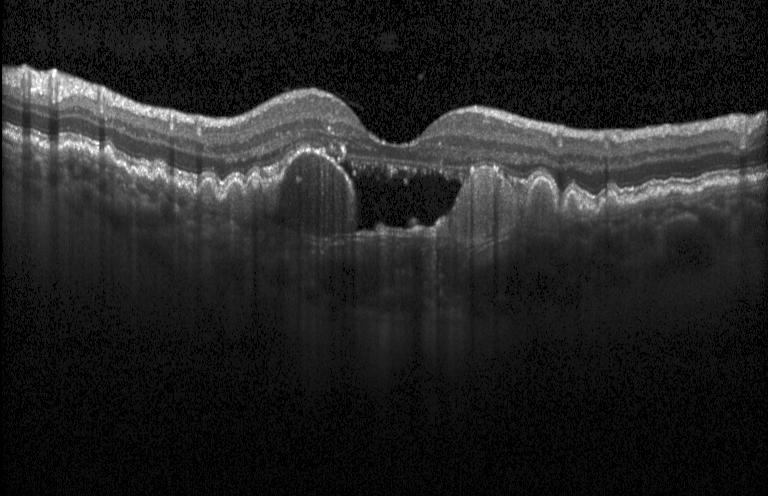 Instrument: Heidelberg Spectralis. Retinal OCT B-scan. Through the macula. SD-OCT — This B-scan demonstrates choroidal neovascularization.